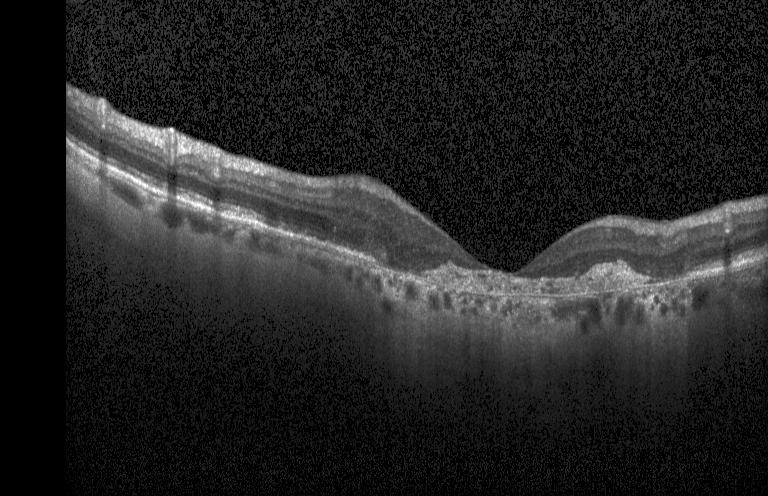 Optical coherence tomography scan.
Diagnosis: CNV.